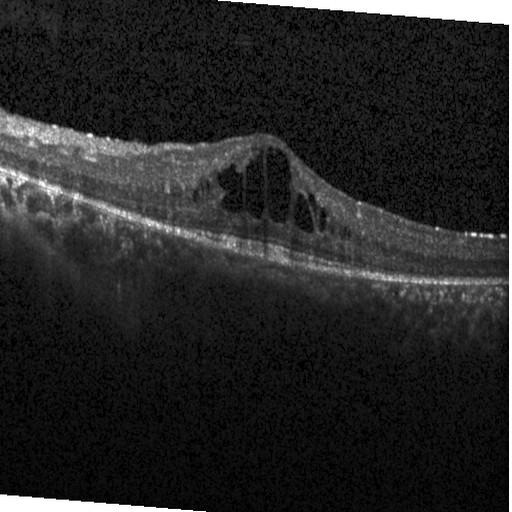 Spectral-domain OCT, retinal OCT cross-section, centered on the fovea, instrument: Heidelberg Spectralis
Impression: diabetic macular edema.